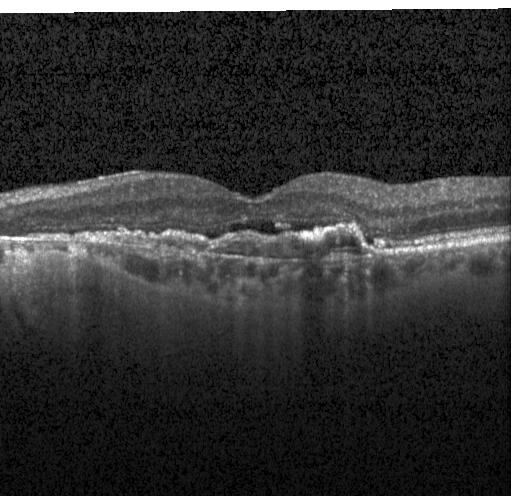

OCT B-scan showing CNV.